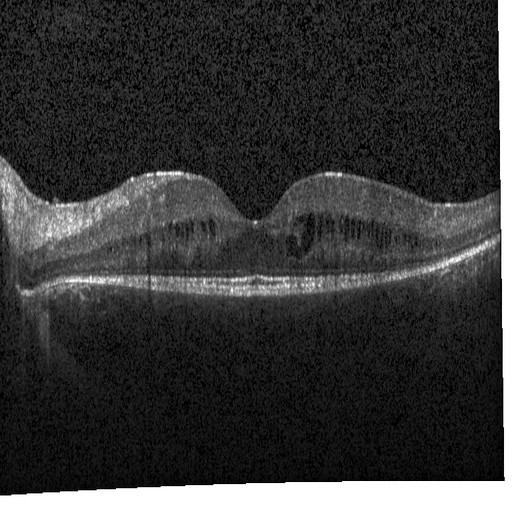 OCT line scan; horizontal scan through the fovea. Diabetic macular edema.